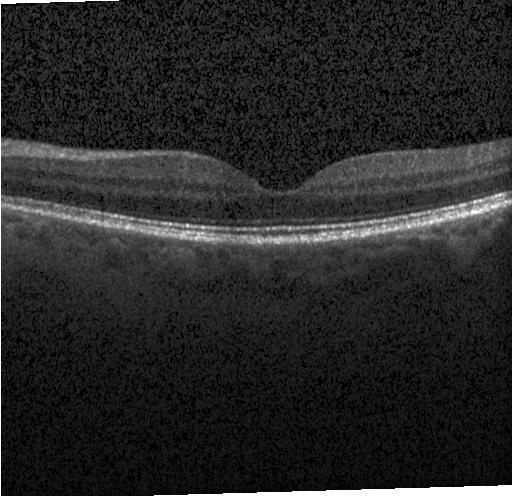 OCT finding: no evidence of choroidal neovascularization, diabetic macular edema, or drusen.